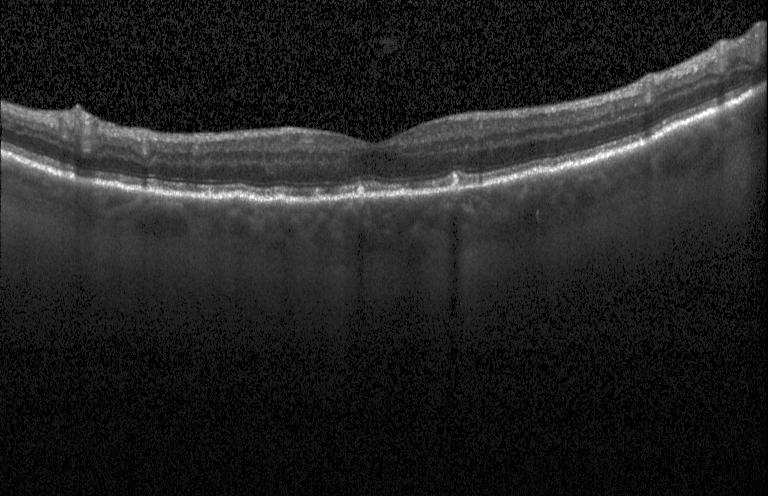

Retinal OCT cross-section showing multiple drusen.